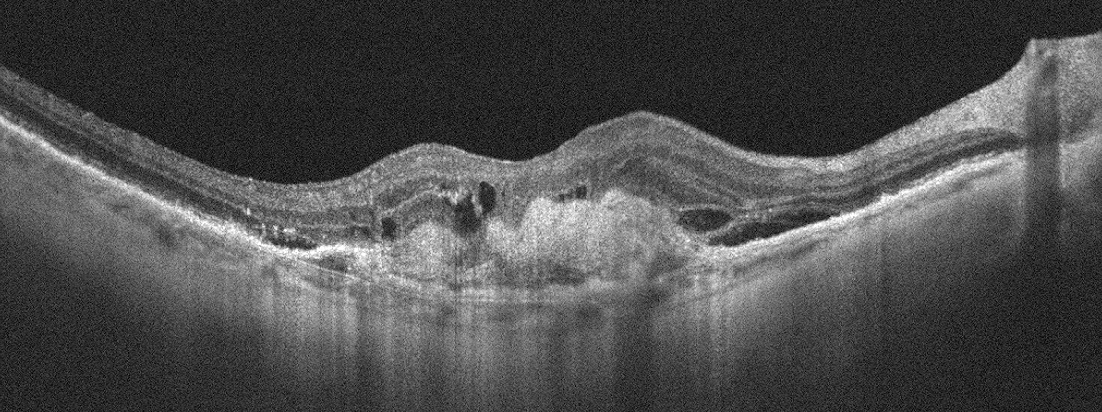

This B-scan demonstrates age-related macular degeneration (AMD).